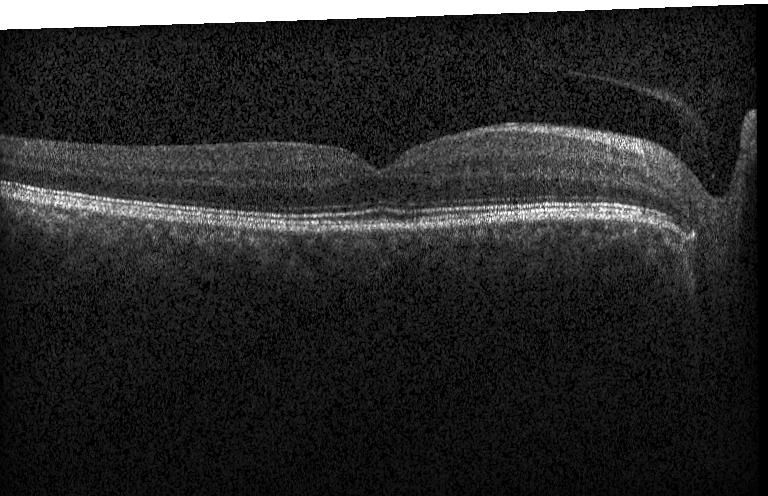
Retinal OCT cross-section; spectral-domain OCT.
Diagnosis: no choroidal neovascularization, no diabetic macular edema, and no drusen.